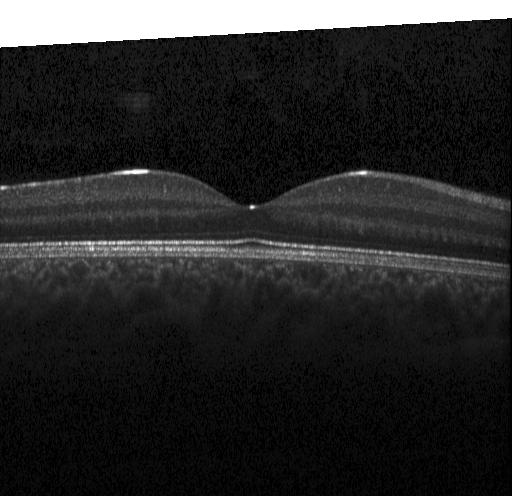

OCT finding: no choroidal neovascularization, no diabetic macular edema, and no drusen.